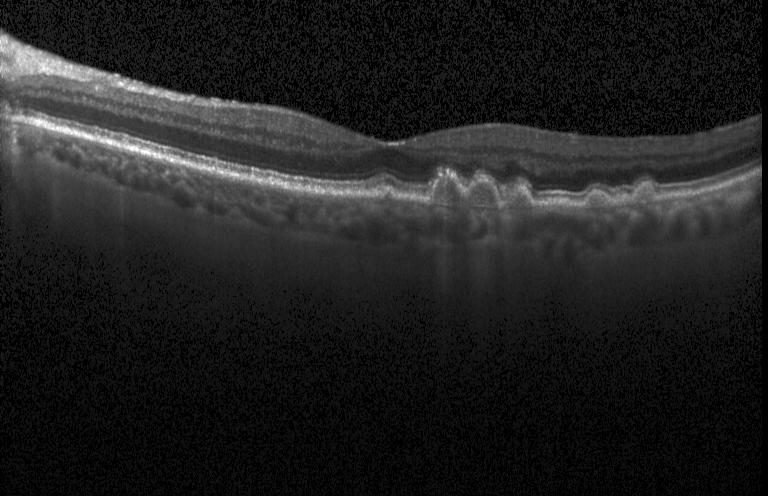

Optical coherence tomography scan — Dx: multiple drusen.